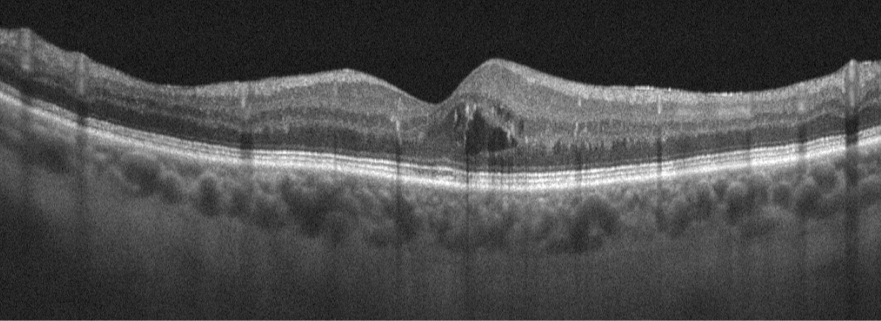 Assessment: DME.